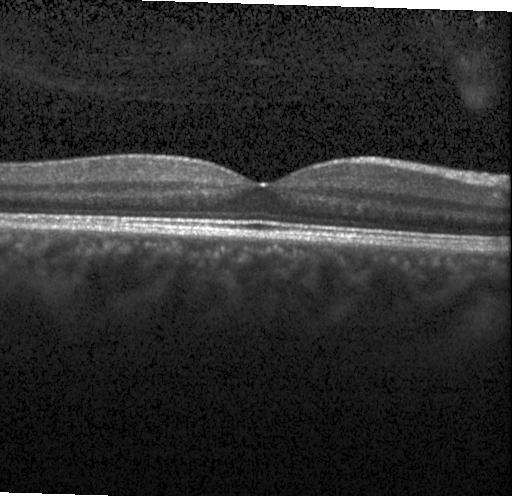

Assessment: neither choroidal neovascularization, diabetic macular edema, nor drusen.